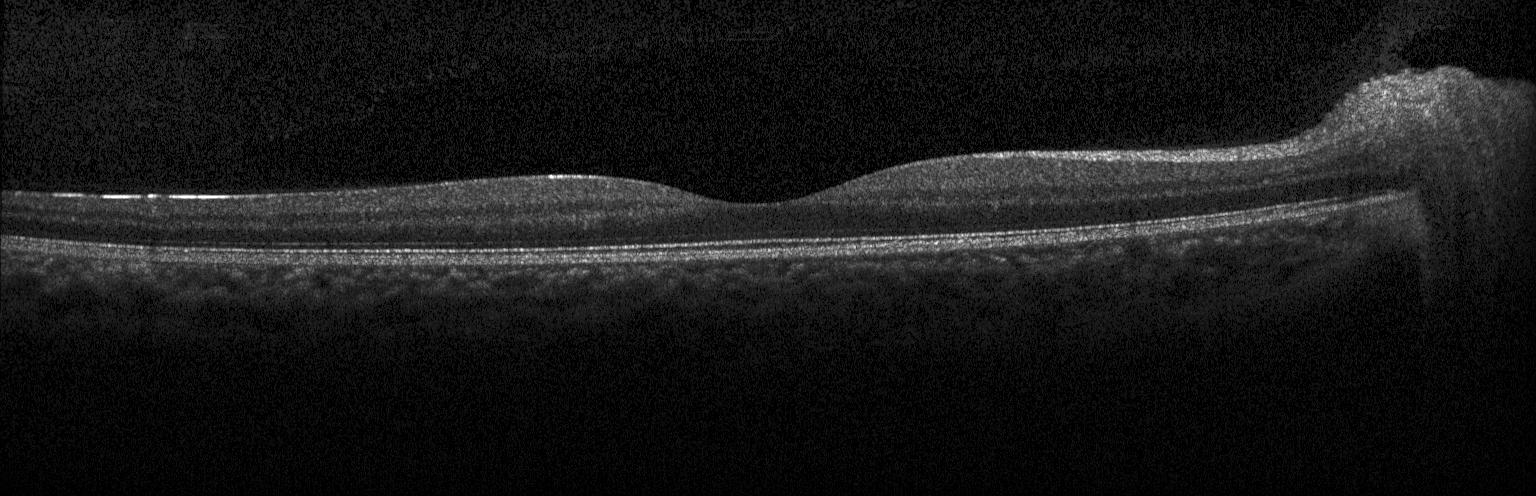 This B-scan demonstrates no choroidal neovascularization, diabetic macular edema, or drusen.